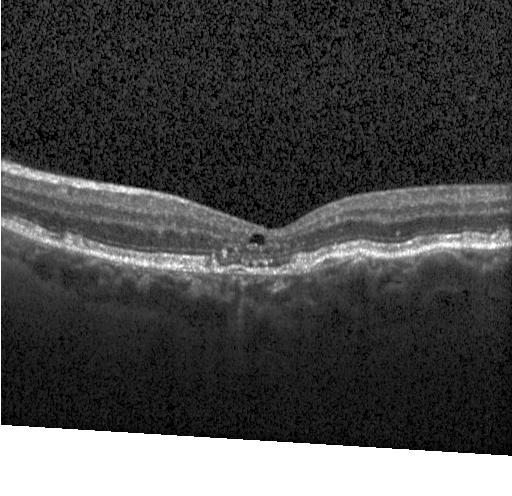
OCT finding: a choroidal neovascular membrane.